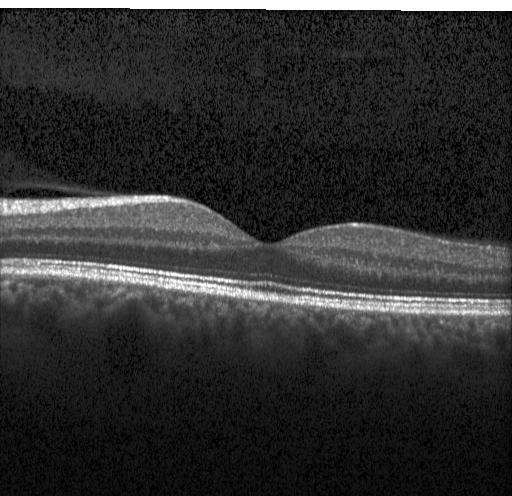 Diagnosis: no choroidal neovascularization, diabetic macular edema, or drusen.